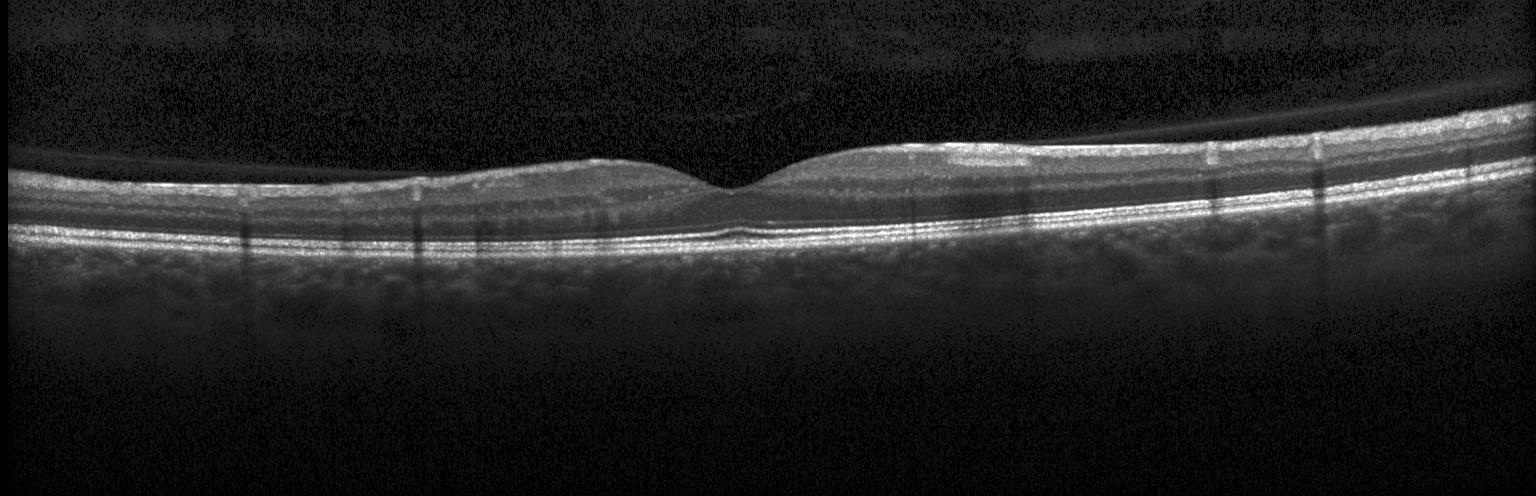
OCT finding: no choroidal neovascularization, no diabetic macular edema, and no drusen.